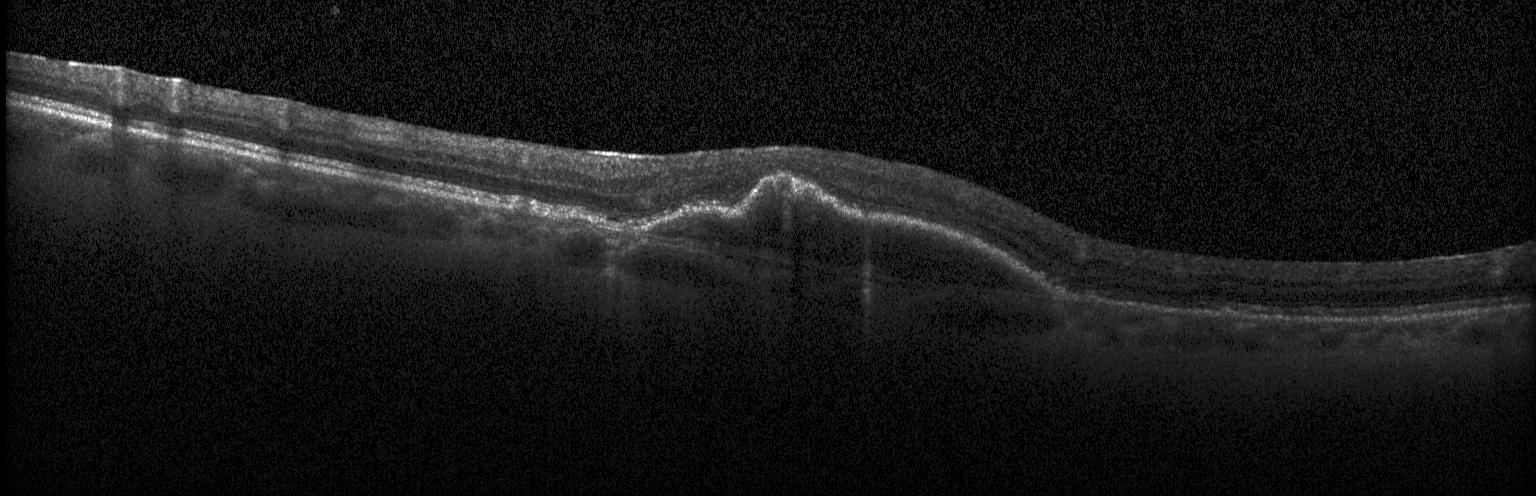 Finding: a choroidal neovascular membrane.